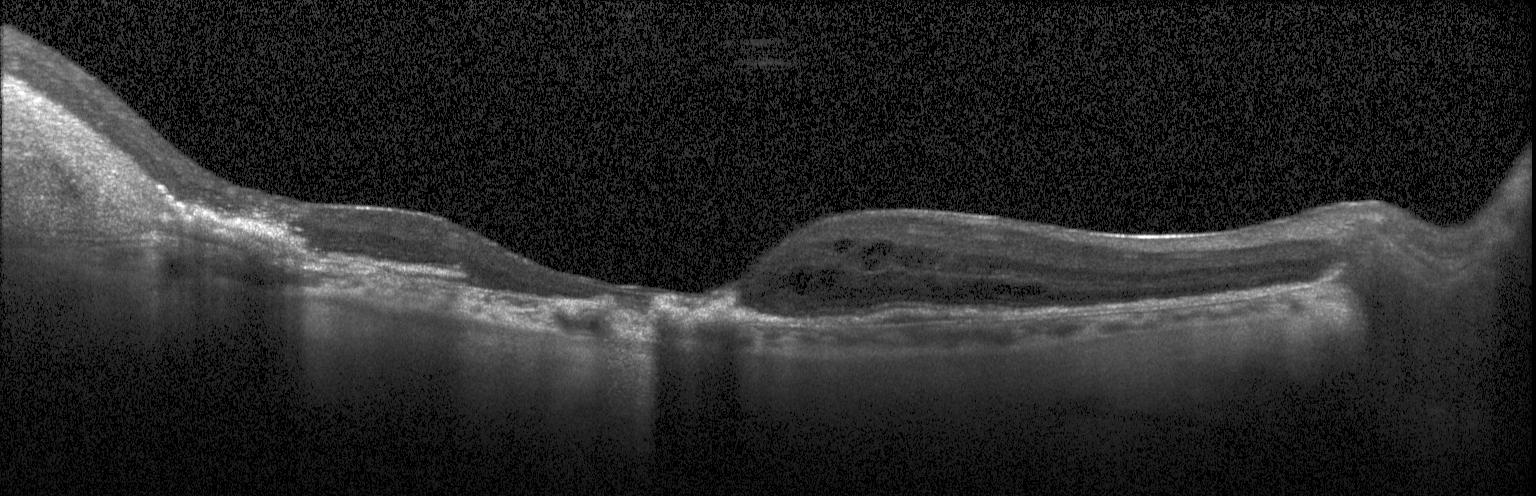

Horizontal scan through the fovea, OCT B-scan, Heidelberg Spectralis OCT system — Impression: a choroidal neovascular membrane.